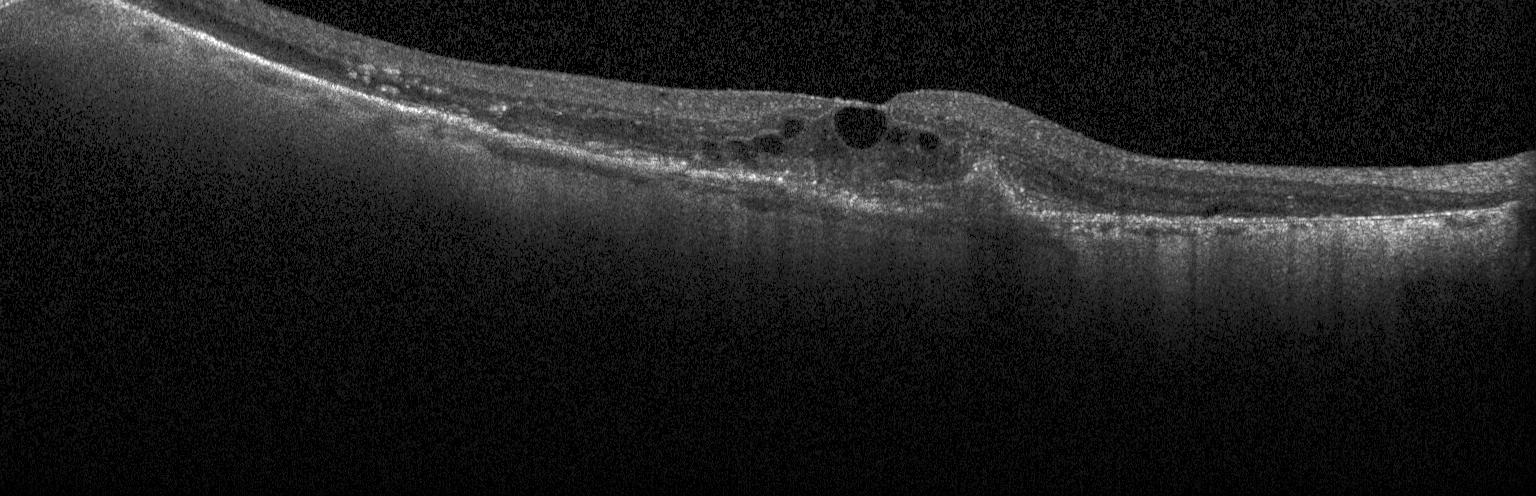

Fovea-centered. Optical coherence tomography B-scan. Finding: choroidal neovascularization (CNV).